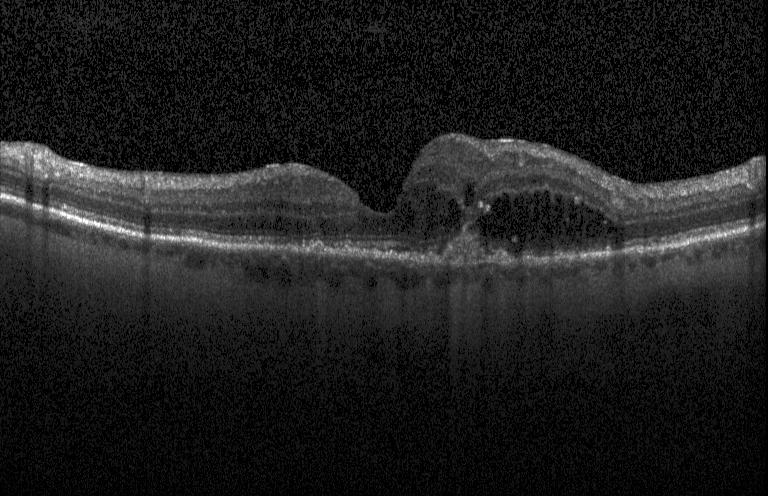

Finding: choroidal neovascularization (CNV).